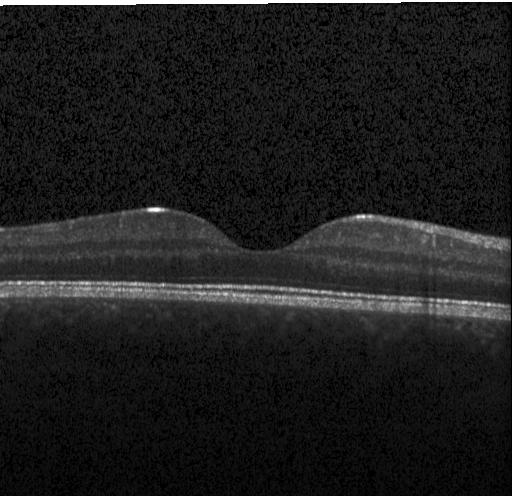 Spectral-domain OCT. Heidelberg Spectralis OCT system. OCT B-scan.
Macular OCT: no CNV, no DME, and no drusen.